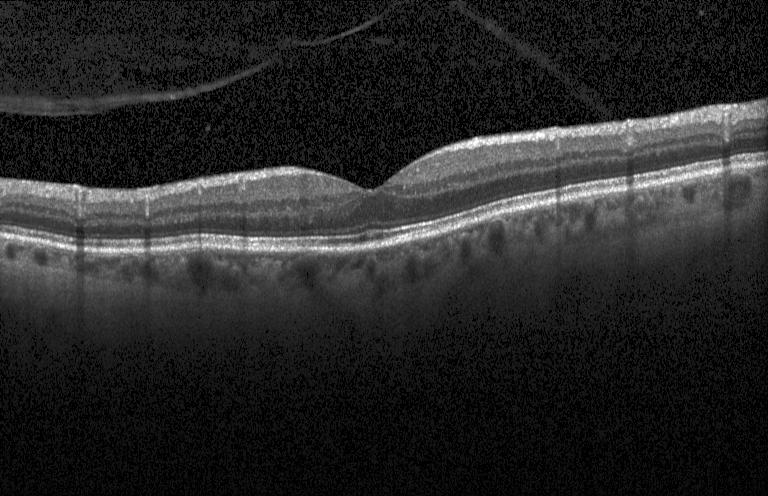

Heidelberg Spectralis OCT system. Spectral-domain optical coherence tomography. Retinal OCT B-scan. Macular scan
Neither CNV, DME, nor drusen.